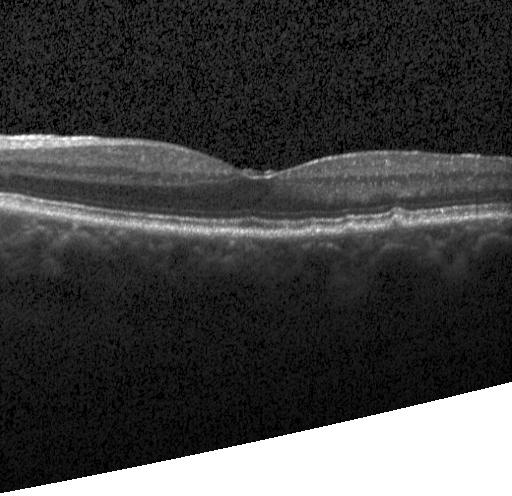
Spectral-domain optical coherence tomography; OCT line scan; centered on the fovea. Assessment: multiple drusen.